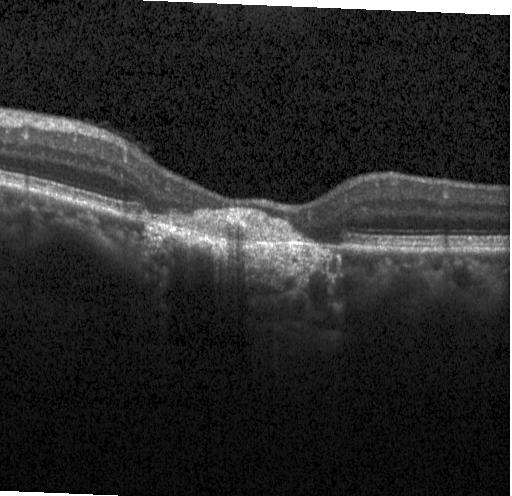

The scan shows CNV.